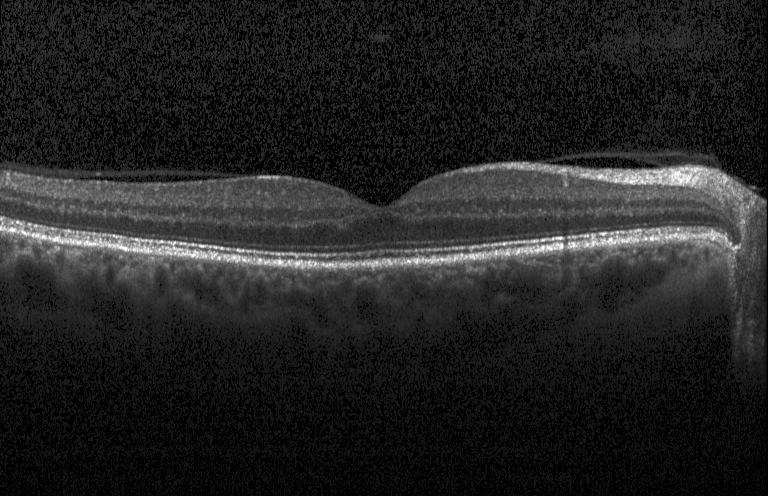

Diagnosis: neither choroidal neovascularization, diabetic macular edema, nor drusen.